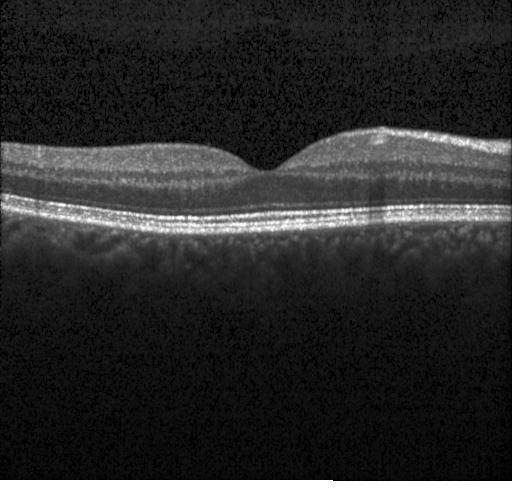

Retinal OCT cross-section — Dx: no choroidal neovascularization, diabetic macular edema, or drusen.